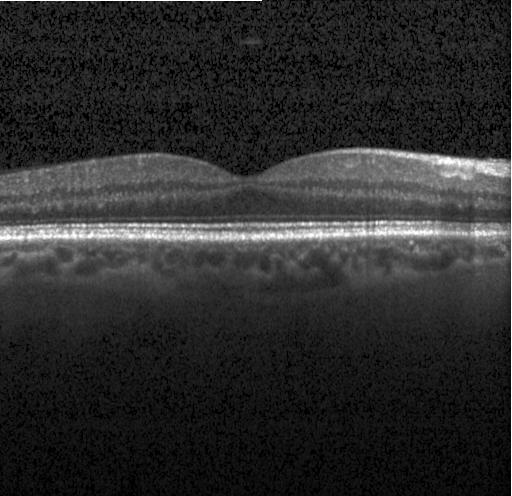 Heidelberg Spectralis · spectral-domain OCT · OCT line scan. Diagnosis: no evidence of choroidal neovascularization, diabetic macular edema, or drusen.